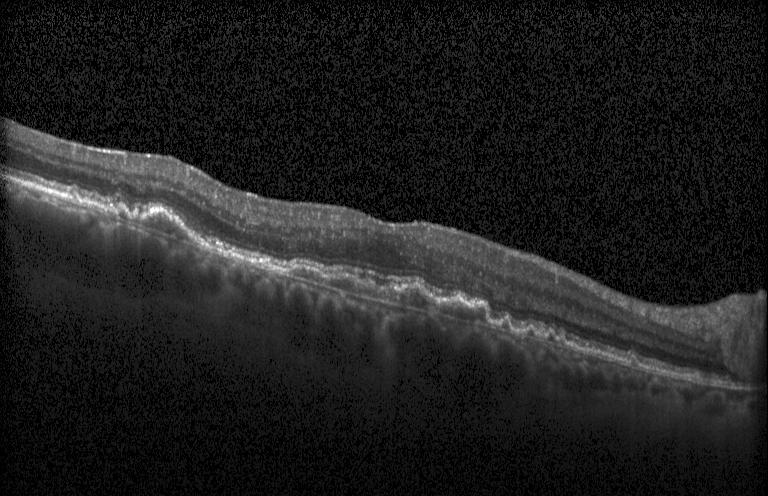

OCT B-scan · SD-OCT.
Diagnosis: choroidal neovascularization.